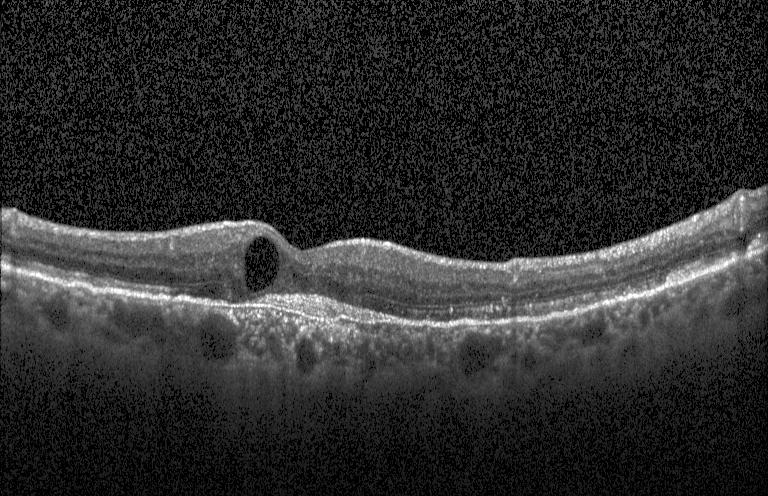

Acquired on a Heidelberg Spectralis, optical coherence tomography B-scan — Impression: a choroidal neovascular membrane.